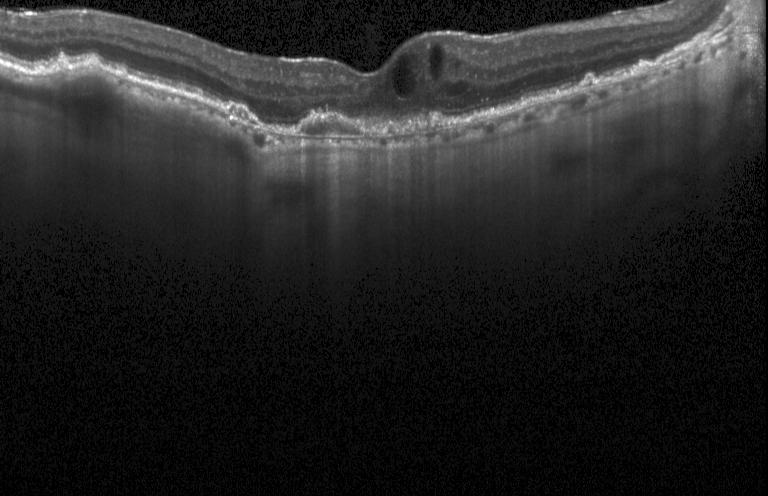
Spectral-domain optical coherence tomography · acquired on a Heidelberg Spectralis · OCT B-scan · centered on the fovea
Impression: a choroidal neovascular membrane.